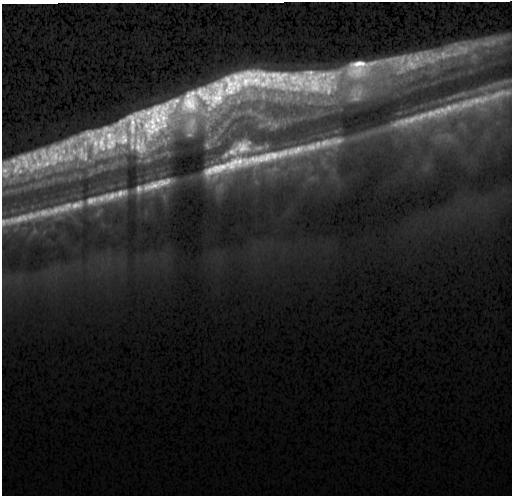

Finding: a choroidal neovascular membrane.